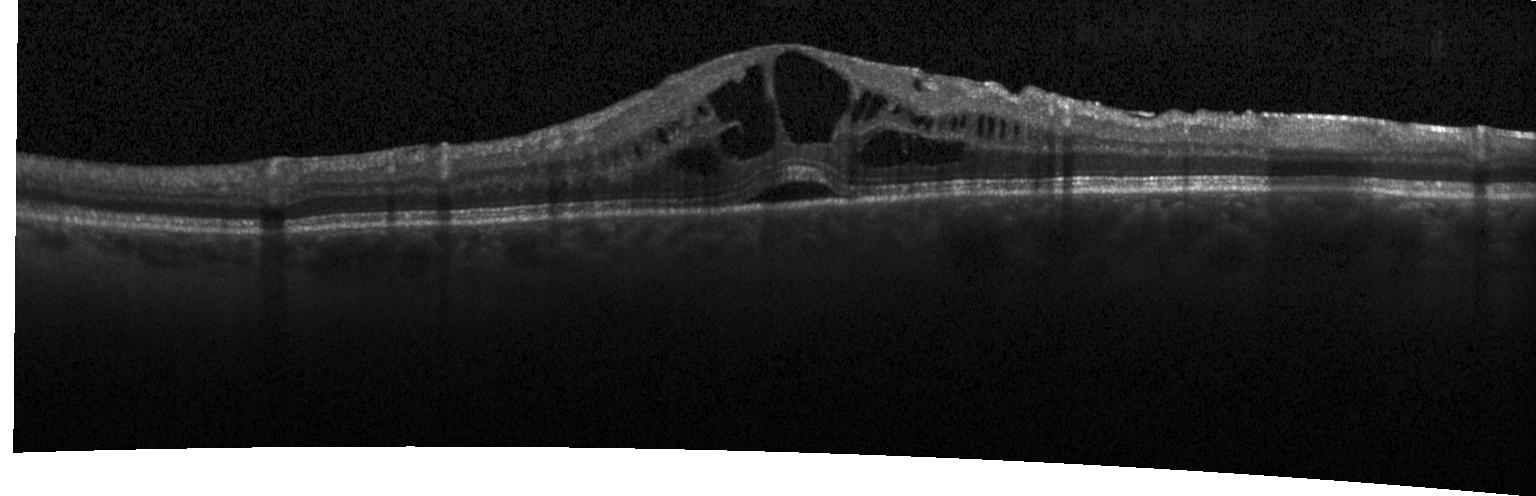 Macular OCT: DME.